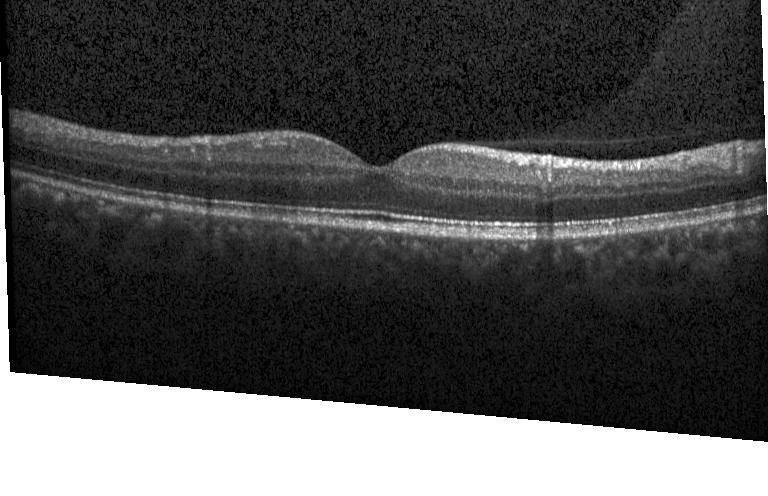 Impression: no choroidal neovascularization, diabetic macular edema, or drusen.